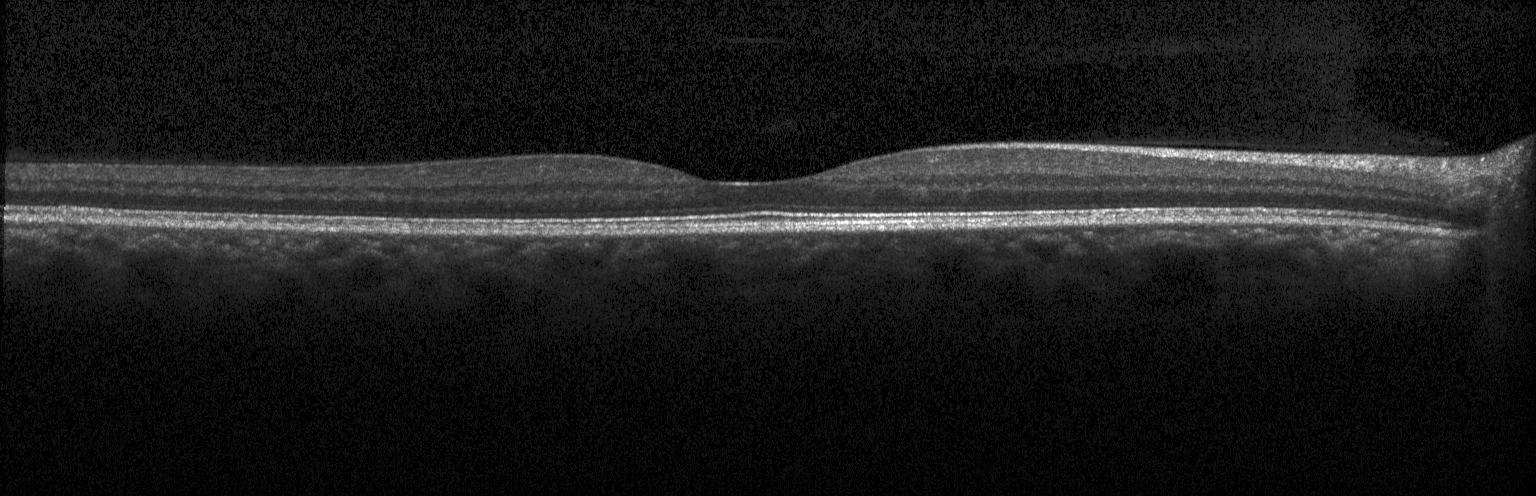
Instrument: Heidelberg Spectralis; spectral-domain OCT; OCT B-scan
The scan shows neither choroidal neovascularization, diabetic macular edema, nor drusen.